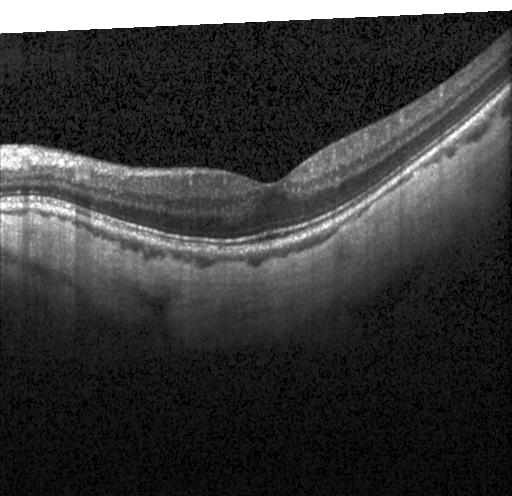 Diagnosis: no CNV, no DME, and no drusen.